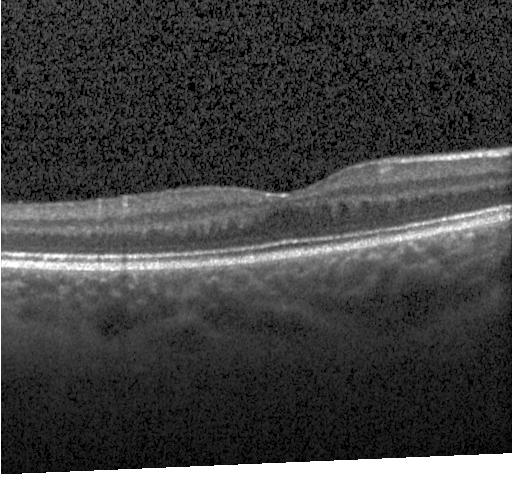

Dx: no evidence of choroidal neovascularization, diabetic macular edema, or drusen.